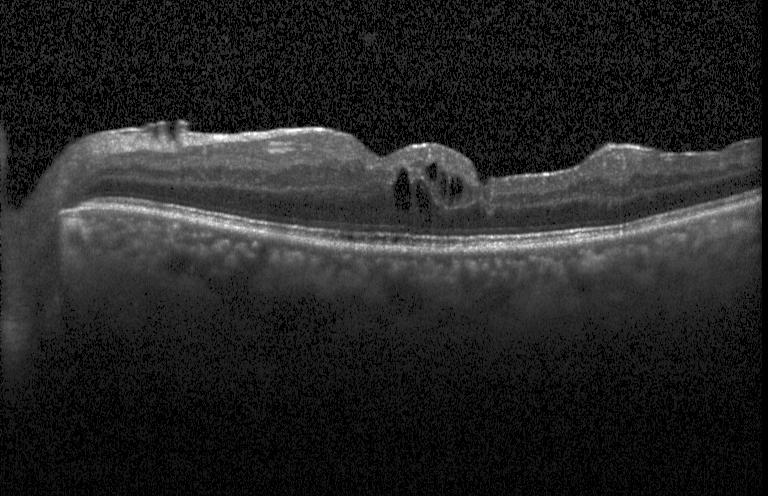
Assessment: diabetic macular edema.